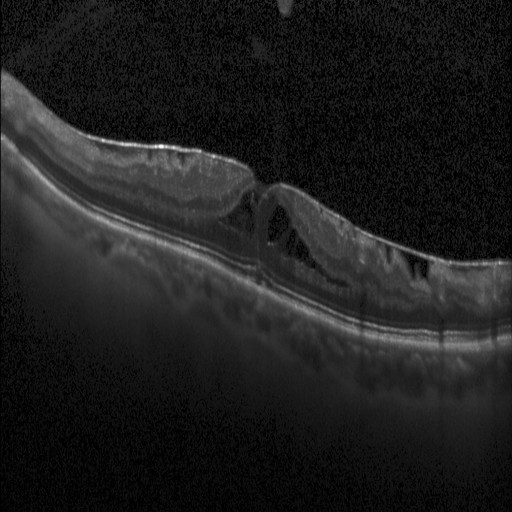 Heidelberg Spectralis, optical coherence tomography B-scan. Impression: diabetic macular edema (DME).